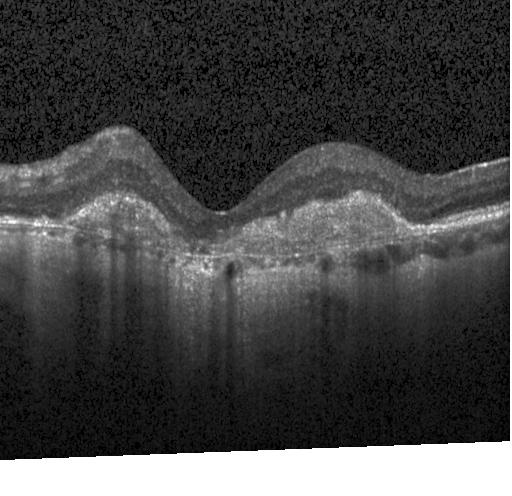
OCT B-scan. Acquired on a Heidelberg Spectralis.
Finding: a choroidal neovascular membrane.